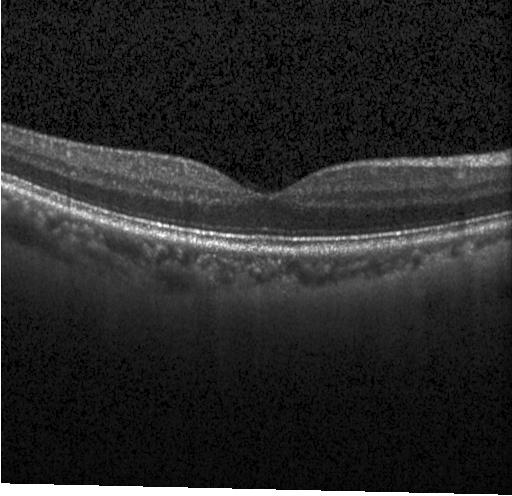

Heidelberg Spectralis OCT system · optical coherence tomography scan · centered on the fovea · SD-OCT. Macular OCT: neither choroidal neovascularization, diabetic macular edema, nor drusen.